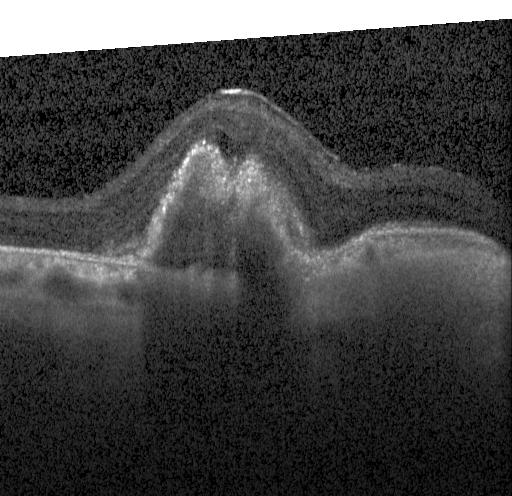 Macular OCT: choroidal neovascularization (CNV).